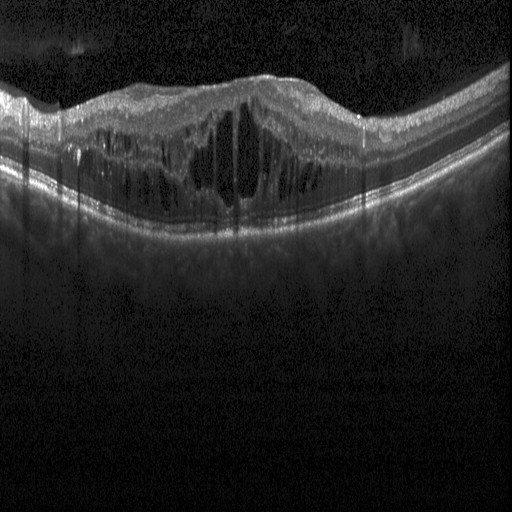
Through the macula; SD-OCT; OCT line scan; instrument: Heidelberg Spectralis.
Diagnosis: diabetic macular edema.